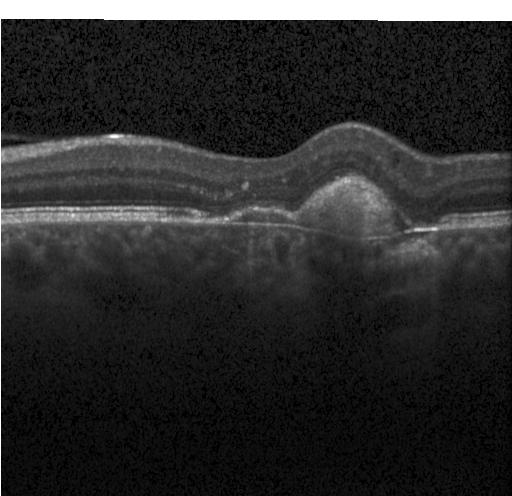
SD-OCT, through the macula, retinal OCT B-scan, acquired on a Heidelberg Spectralis — Assessment: a choroidal neovascular membrane.